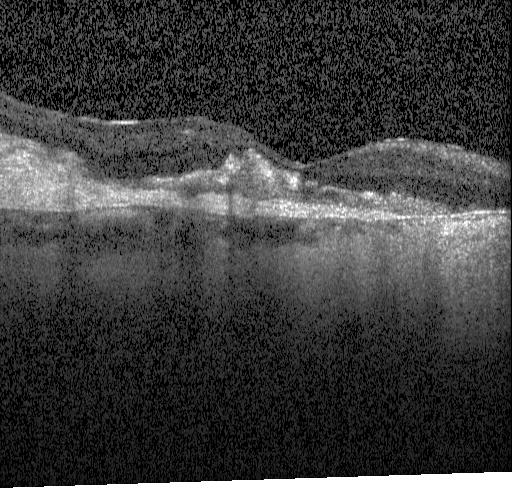

Finding: a choroidal neovascular membrane.